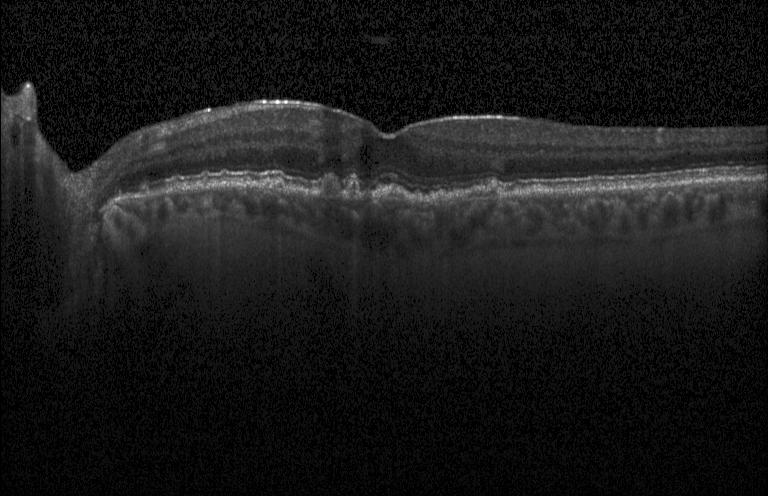
Finding: multiple drusen.